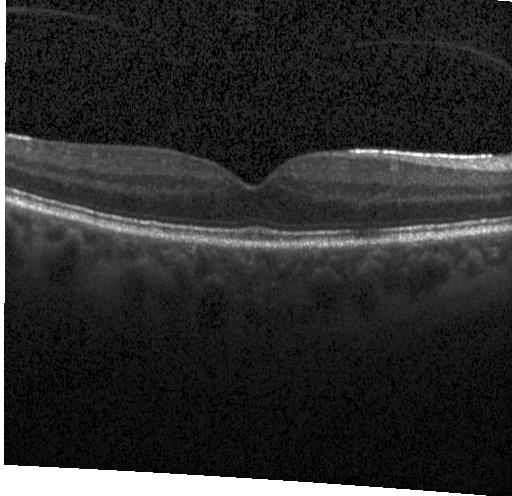

OCT finding: no evidence of choroidal neovascularization, diabetic macular edema, or drusen.